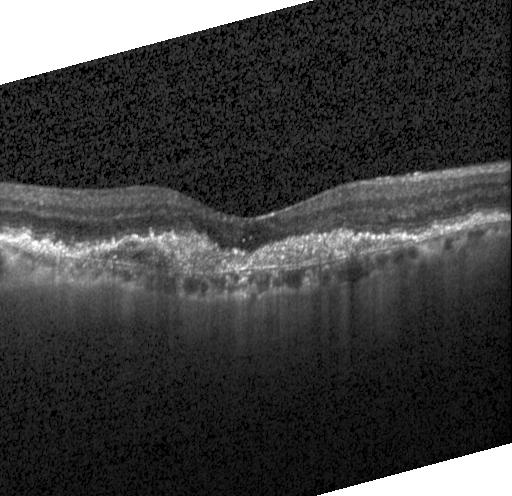
Heidelberg Spectralis OCT system, OCT B-scan
Dx: choroidal neovascularization.